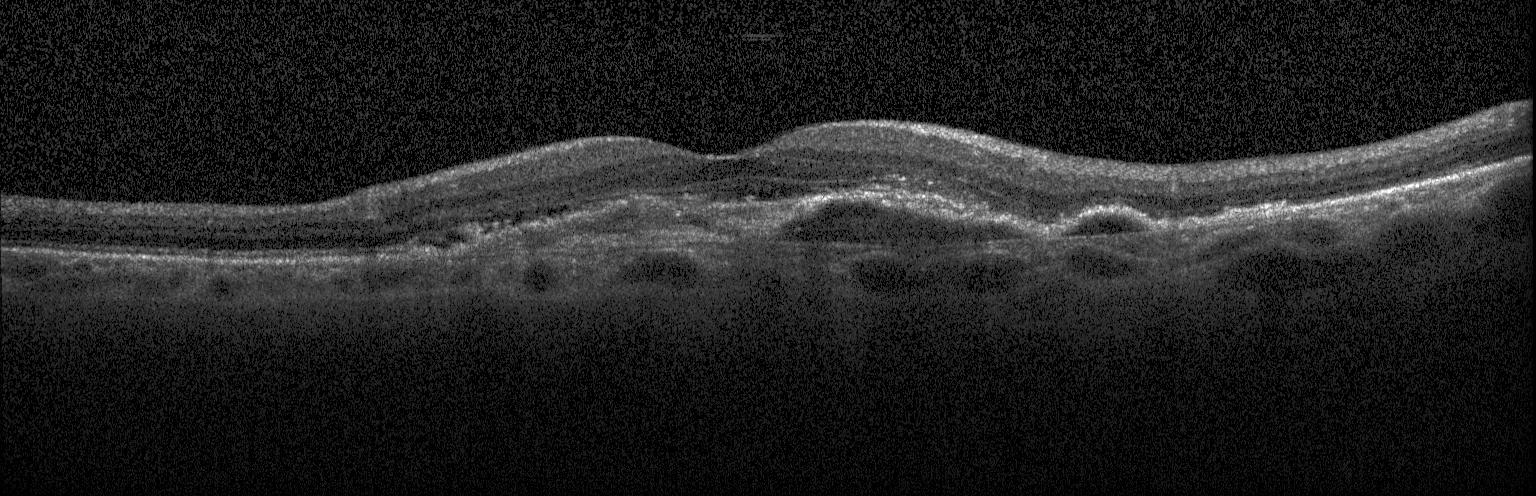
A choroidal neovascular membrane.